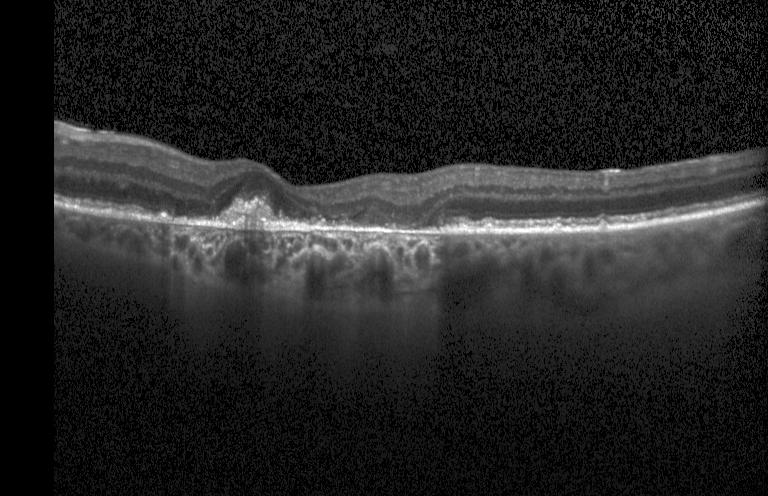

SD-OCT; optical coherence tomography scan
Dx: a choroidal neovascular membrane.